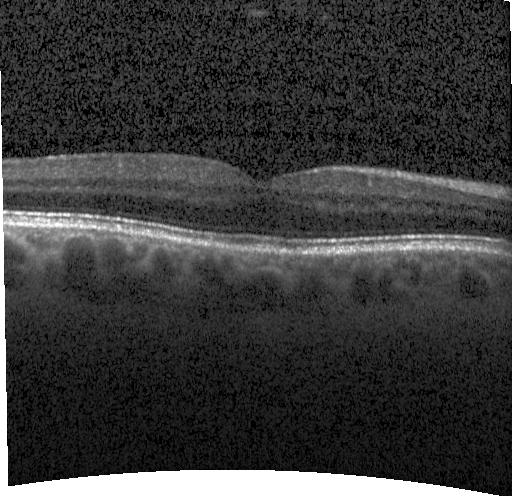 SD-OCT. Optical coherence tomography scan
Diagnosis: neither CNV, DME, nor drusen.